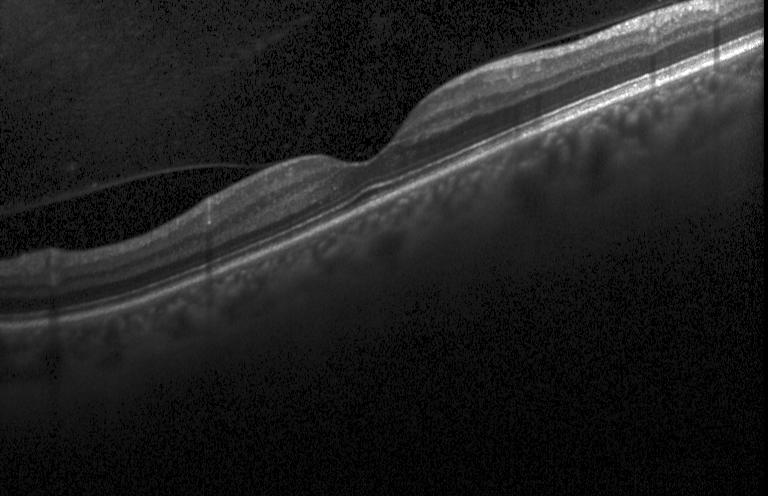
Instrument: Heidelberg Spectralis. SD-OCT. Retinal OCT cross-section.
Impression: neither choroidal neovascularization, diabetic macular edema, nor drusen.